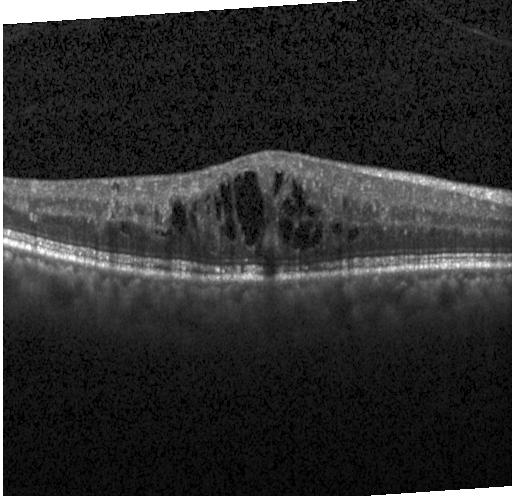
Retinal OCT B-scan. Diagnosis: DME.